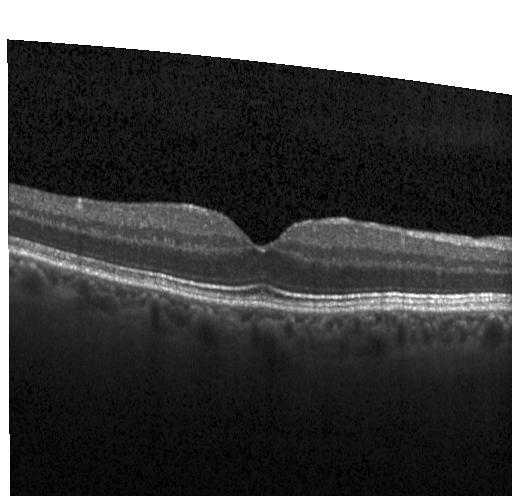 Optical coherence tomography scan. Through the macula. SD-OCT.
OCT finding: no evidence of CNV, DME, or drusen.